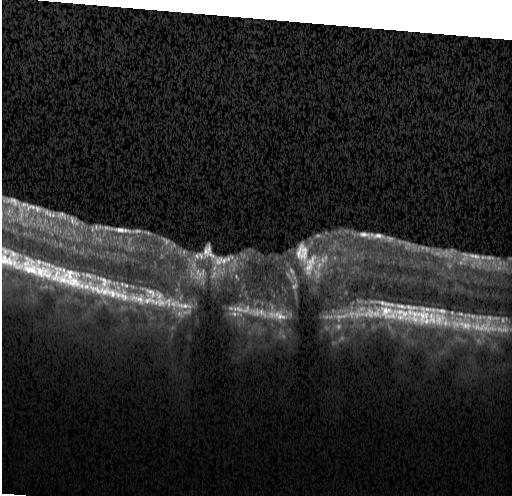 Macular scan; Heidelberg Spectralis; retinal OCT cross-section; SD-OCT
Impression: choroidal neovascularization (CNV).